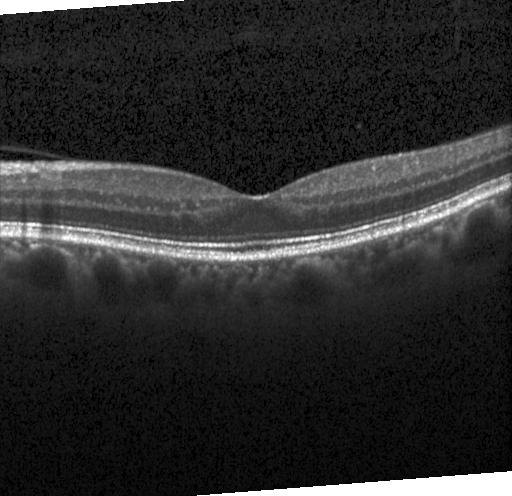

Dx: no choroidal neovascularization, diabetic macular edema, or drusen.